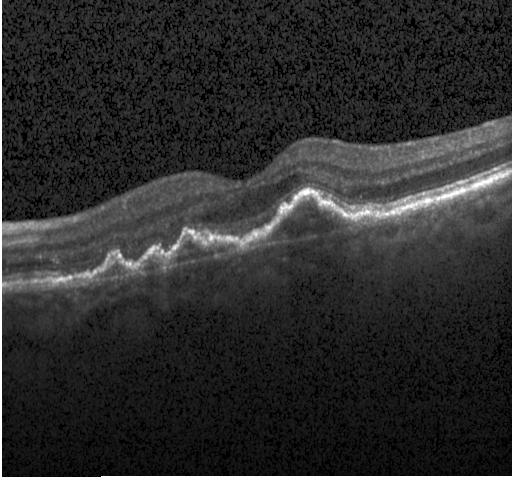

Optical coherence tomography B-scan — OCT finding: a choroidal neovascular membrane.